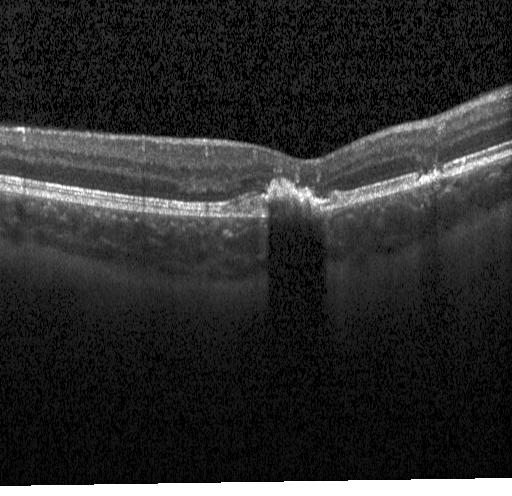

SD-OCT · optical coherence tomography B-scan.
Macular OCT: a choroidal neovascular membrane.